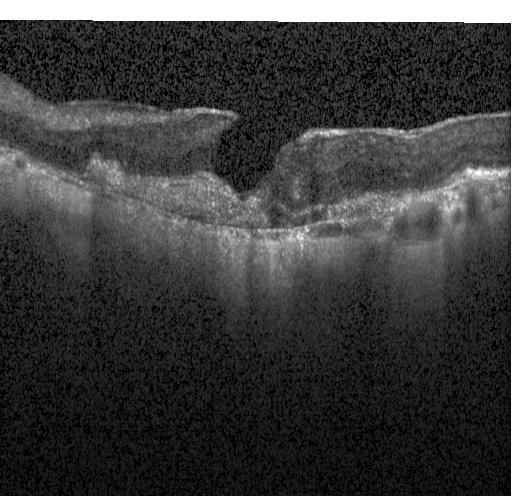

SD-OCT · instrument: Heidelberg Spectralis · optical coherence tomography B-scan
Finding: a choroidal neovascular membrane.